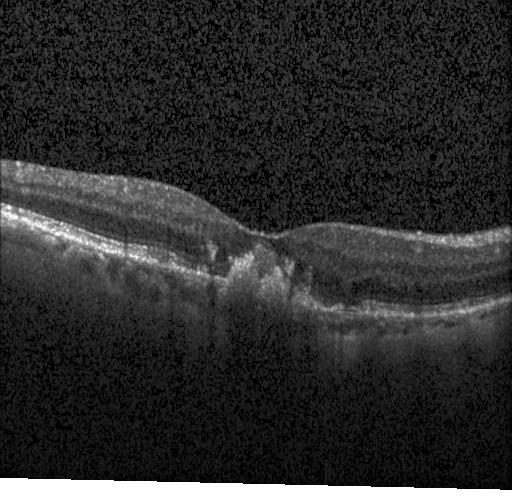
Acquired on a Heidelberg Spectralis, optical coherence tomography scan, spectral-domain optical coherence tomography, centered on the fovea — Diagnosis: a choroidal neovascular membrane.